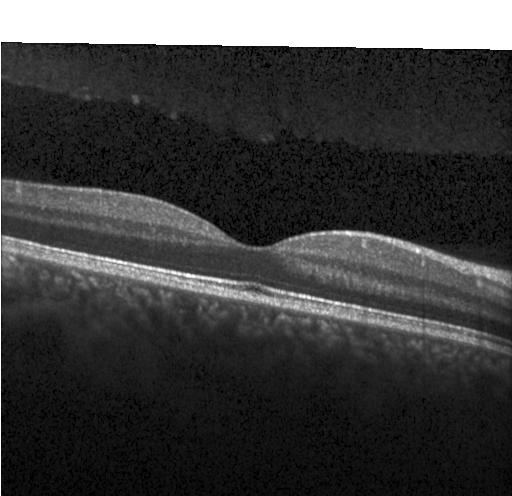 Fovea-centered · optical coherence tomography B-scan · spectral-domain optical coherence tomography.
Dx: no choroidal neovascularization, no diabetic macular edema, and no drusen.